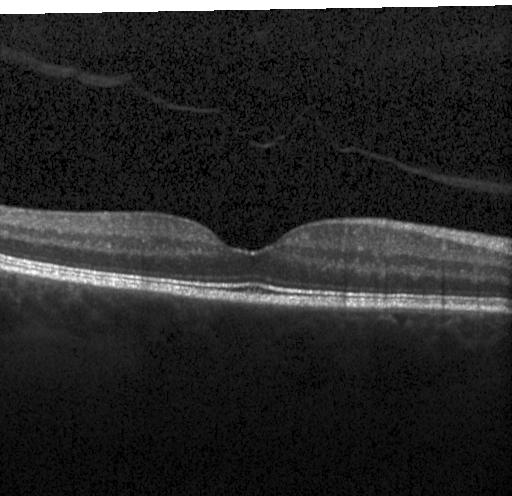 Optical coherence tomography scan; acquired on a Heidelberg Spectralis; SD-OCT. Finding: no choroidal neovascularization, no diabetic macular edema, and no drusen.